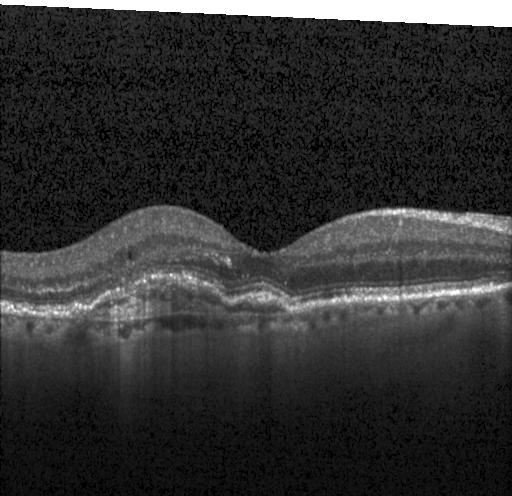 Optical coherence tomography B-scan, centered on the fovea, Heidelberg Spectralis — This B-scan demonstrates a choroidal neovascular membrane.